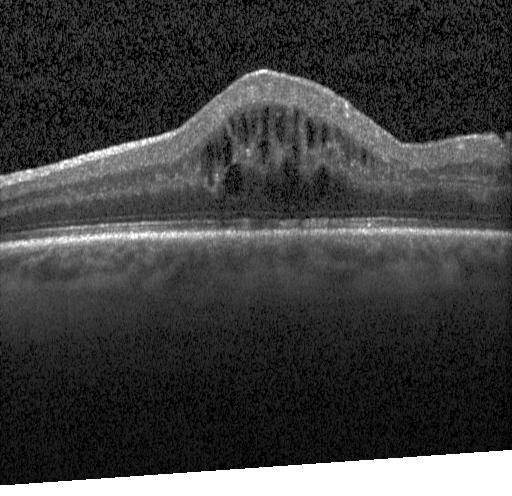
OCT finding: diabetic macular edema (DME).